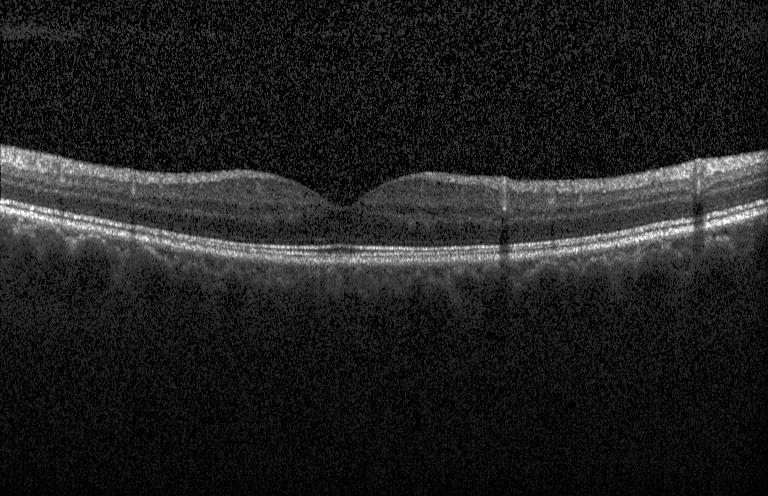

OCT line scan. Fovea-centered. Acquired on a Heidelberg Spectralis
The scan shows no choroidal neovascularization, no diabetic macular edema, and no drusen.